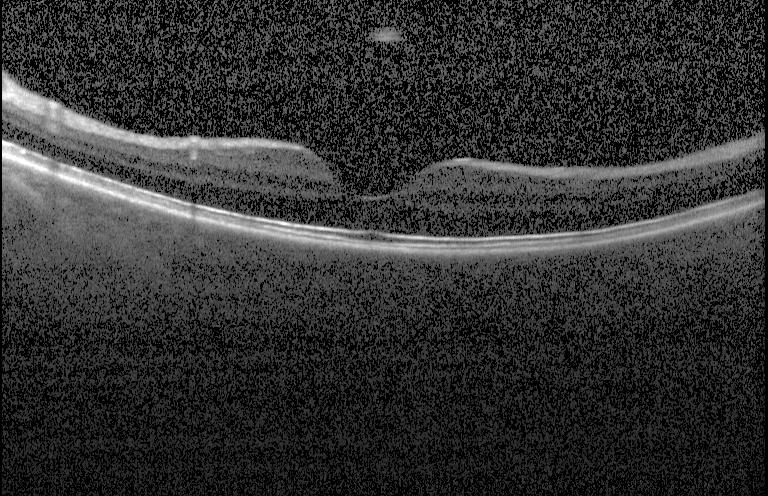

Heidelberg Spectralis OCT system; OCT B-scan.
OCT finding: no choroidal neovascularization, no diabetic macular edema, and no drusen.